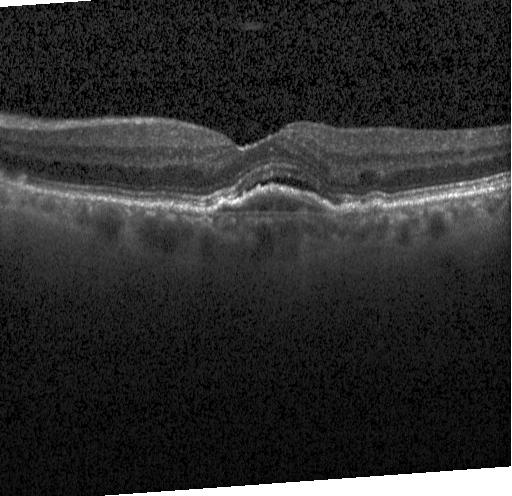

Macular OCT demonstrating a choroidal neovascular membrane.